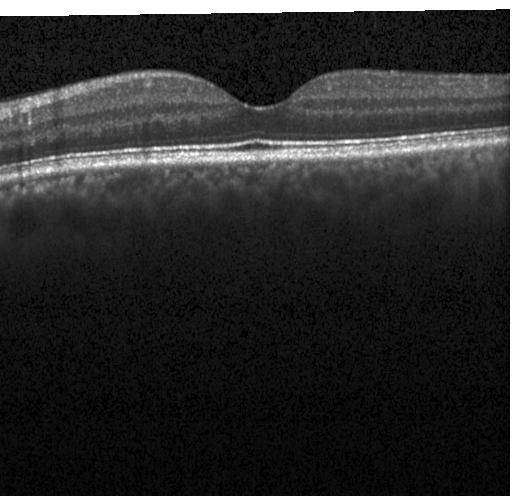 Retinal OCT B-scan · Heidelberg Spectralis OCT system.
Diagnosis: no choroidal neovascularization, no diabetic macular edema, and no drusen.